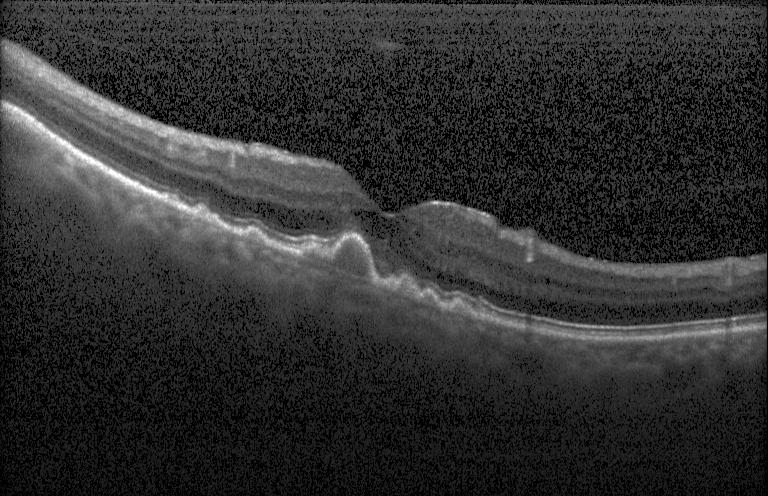

Finding: sub-RPE drusenoid deposits.